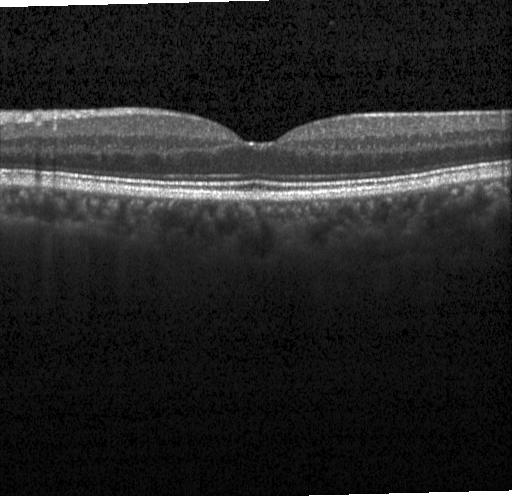

Finding: no evidence of choroidal neovascularization, diabetic macular edema, or drusen.